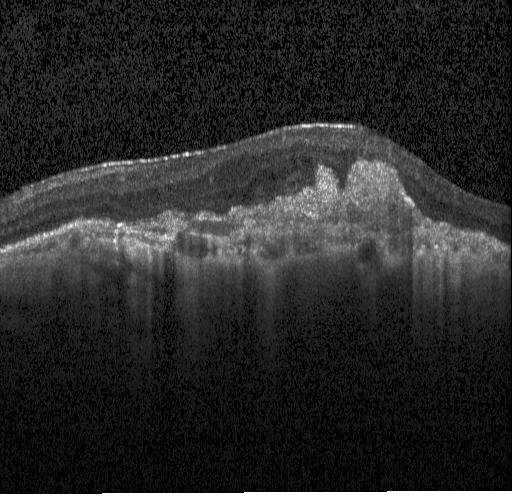
Dx: a choroidal neovascular membrane.